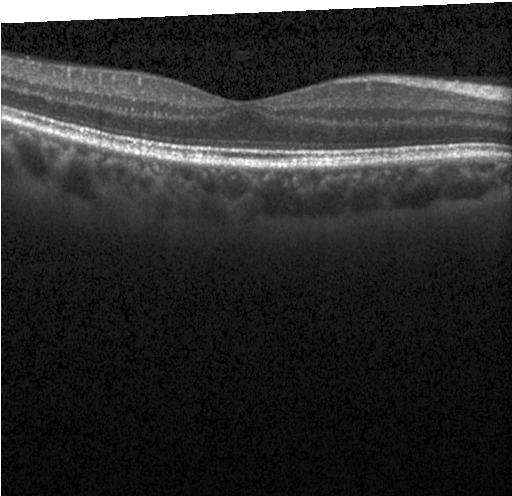 OCT line scan, Heidelberg Spectralis, SD-OCT. Diagnosis: no CNV, no DME, and no drusen.